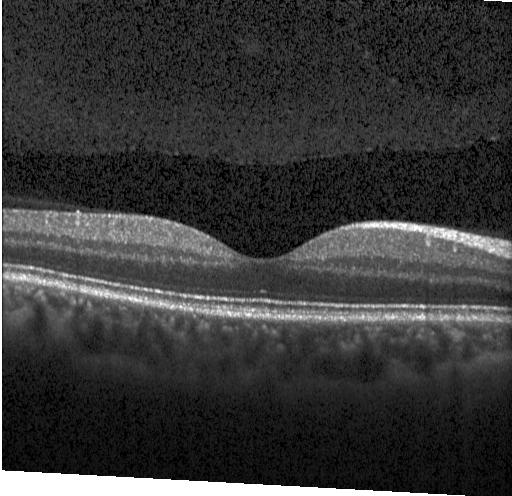

Diagnosis: no choroidal neovascularization, diabetic macular edema, or drusen.